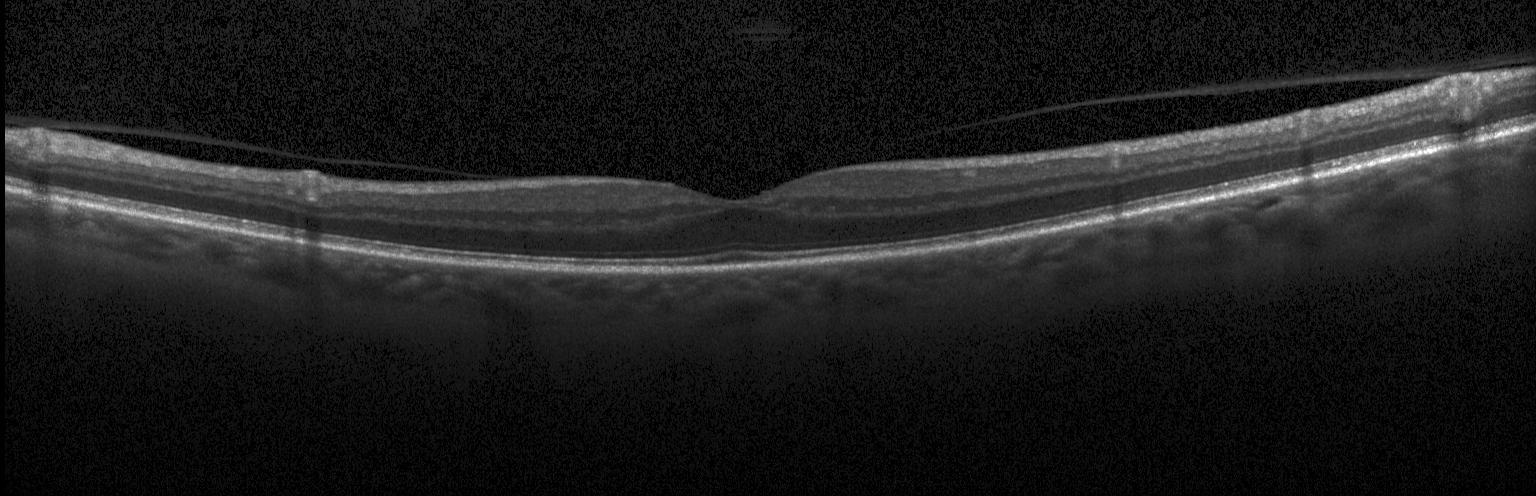
Retinal OCT cross-section. The scan shows no evidence of CNV, DME, or drusen.